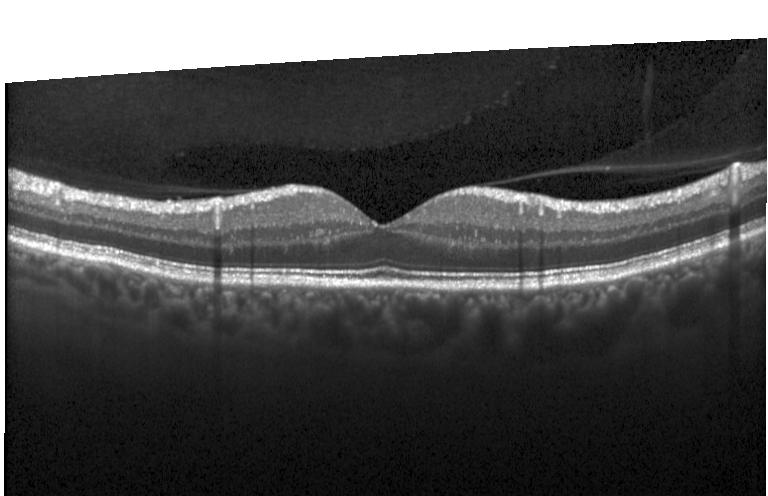

OCT B-scan showing no evidence of choroidal neovascularization, diabetic macular edema, or drusen.